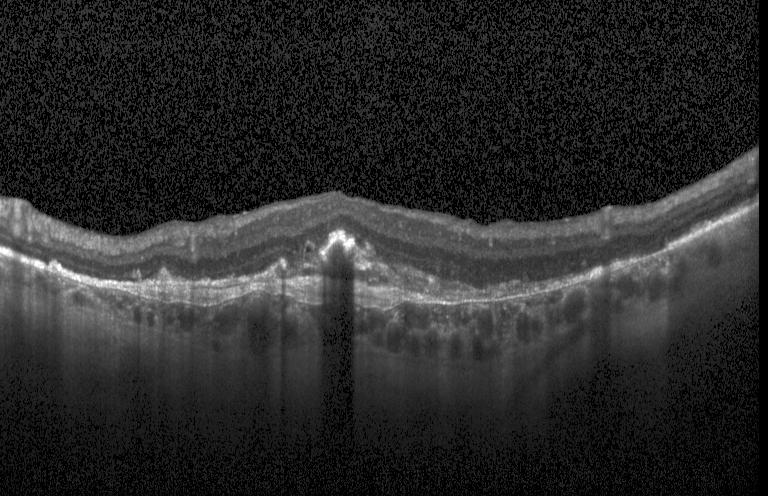
Macular OCT demonstrating CNV.